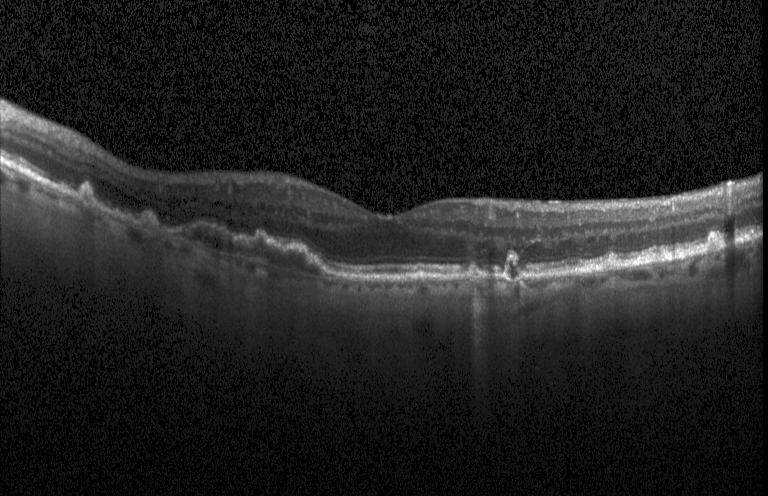

Optical coherence tomography B-scan · Heidelberg Spectralis OCT system · SD-OCT · macular scan — Impression: a choroidal neovascular membrane.